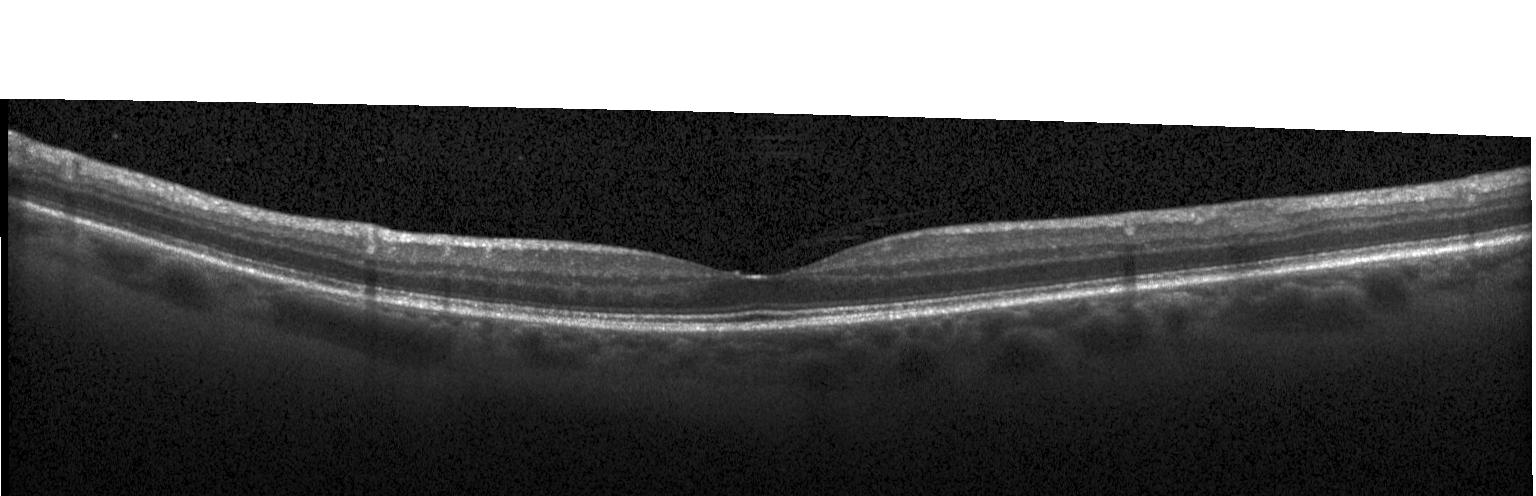 OCT finding: no evidence of choroidal neovascularization, diabetic macular edema, or drusen.